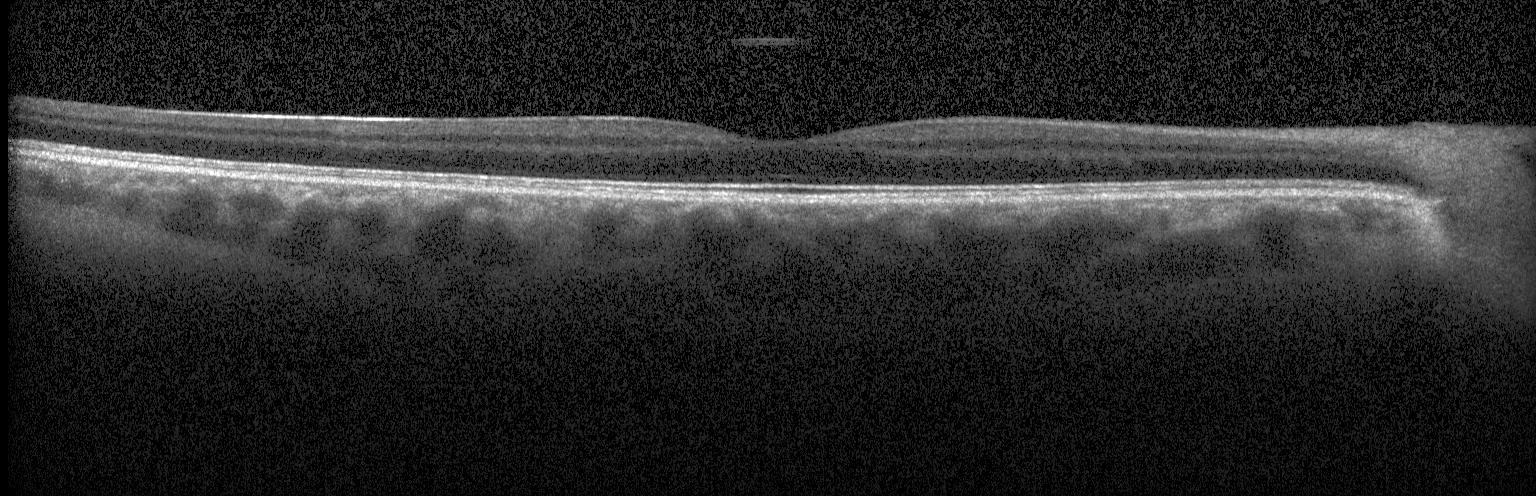
Macular scan. Retinal OCT cross-section — Impression: no choroidal neovascularization, diabetic macular edema, or drusen.